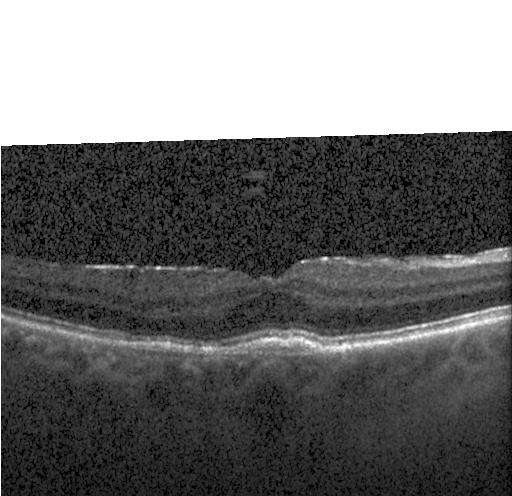 Fovea-centered; optical coherence tomography B-scan — Diagnosis: a choroidal neovascular membrane.